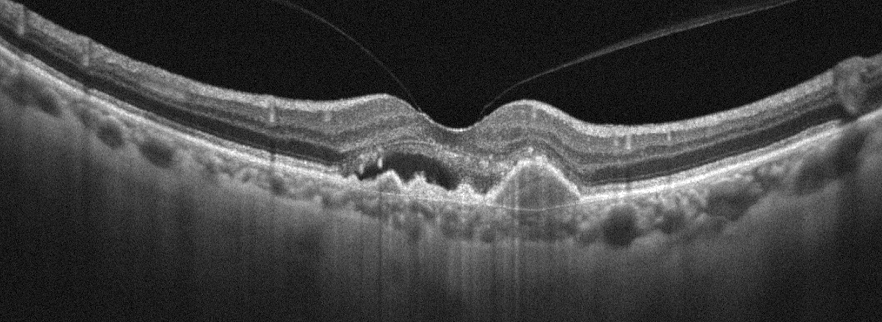 Retinal OCT B-scan; instrument: Optovue Avanti RTVue XR — Diagnosis: age-related macular degeneration.